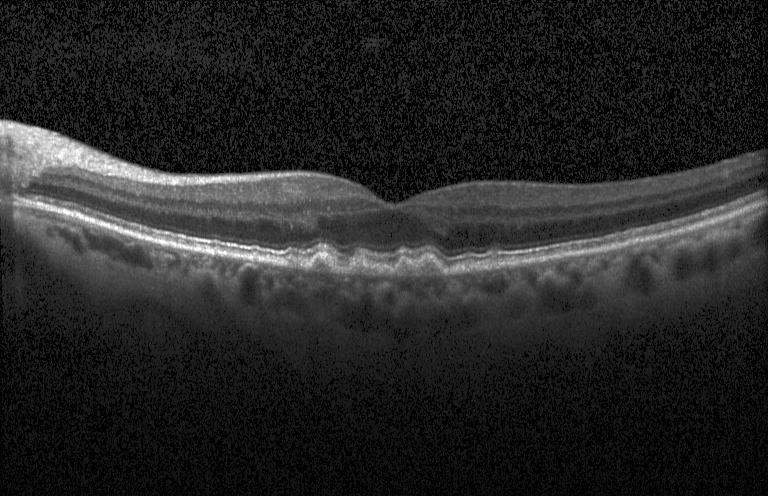 Spectral-domain optical coherence tomography; Heidelberg Spectralis OCT system; OCT B-scan; centered on the fovea — OCT finding: drusen.